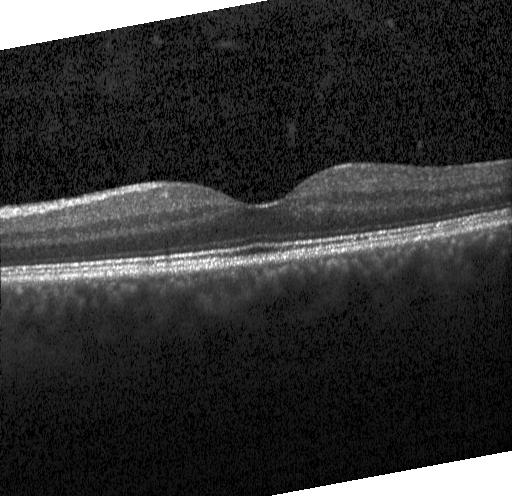 Optical coherence tomography scan.
Macular OCT: no evidence of CNV, DME, or drusen.